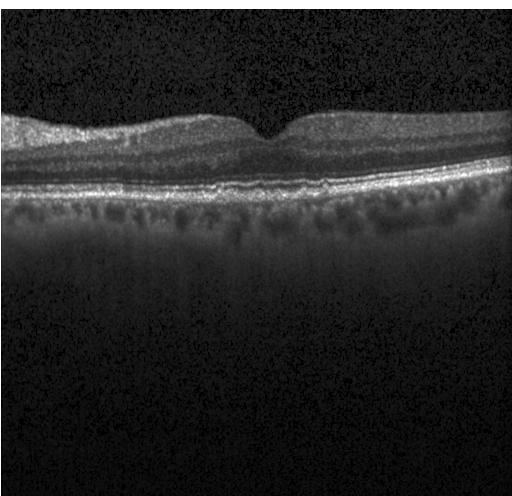 Optical coherence tomography scan; horizontal scan through the fovea; acquired on a Heidelberg Spectralis; SD-OCT.
Assessment: sub-RPE drusenoid deposits.